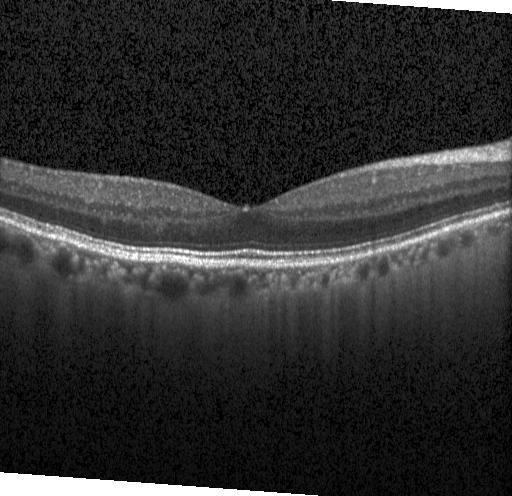 Diagnosis: no choroidal neovascularization, diabetic macular edema, or drusen.